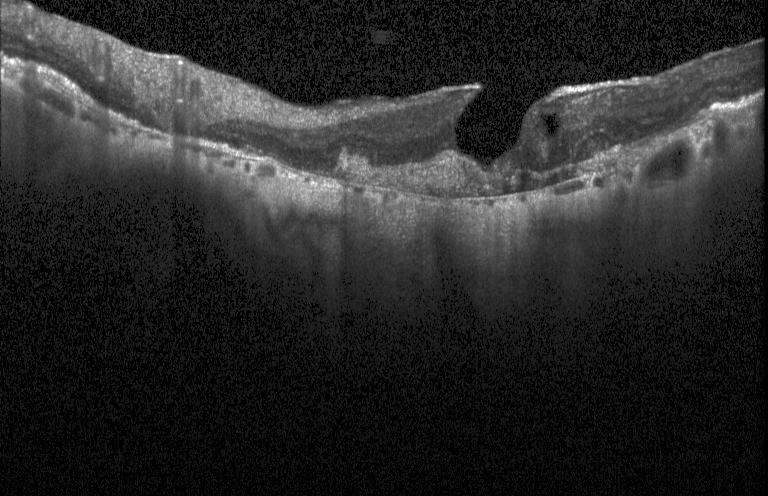 A choroidal neovascular membrane.